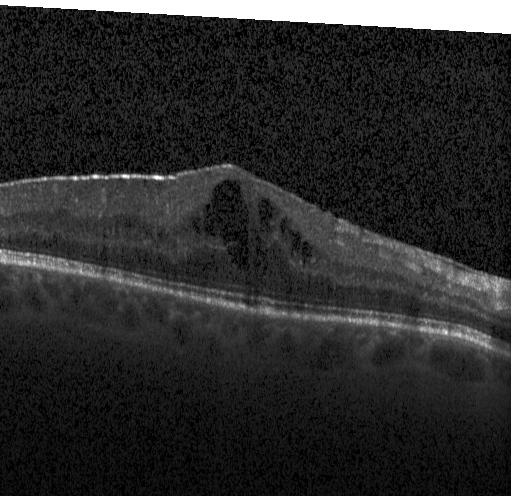

Optical coherence tomography B-scan.
OCT finding: diabetic macular edema.